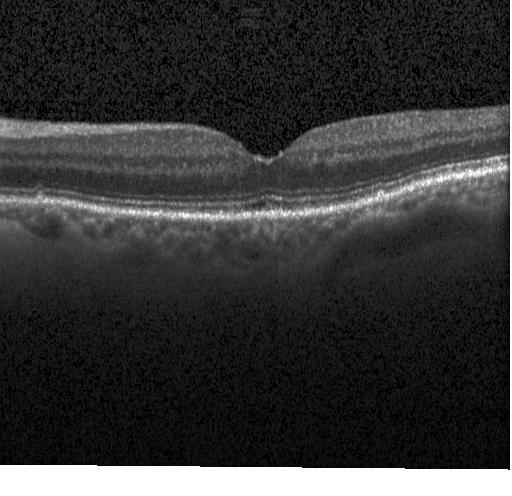 Retinal OCT B-scan. Heidelberg Spectralis OCT system. Macular scan. Macular OCT: multiple drusen.